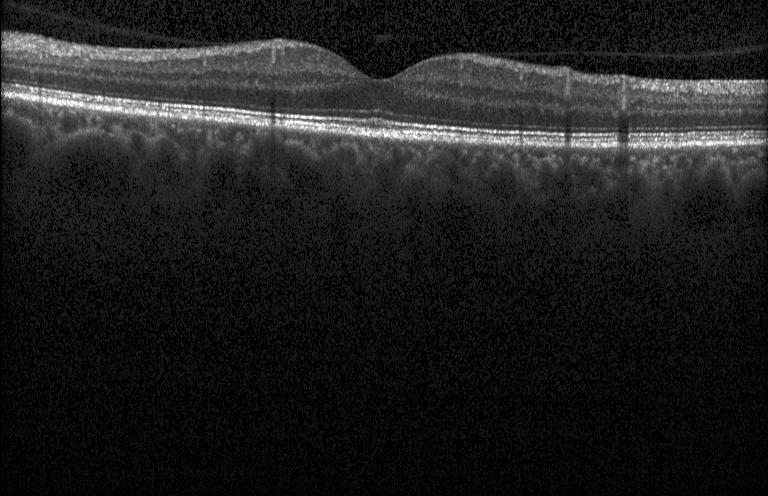 Optical coherence tomography B-scan.
Impression: no evidence of choroidal neovascularization, diabetic macular edema, or drusen.